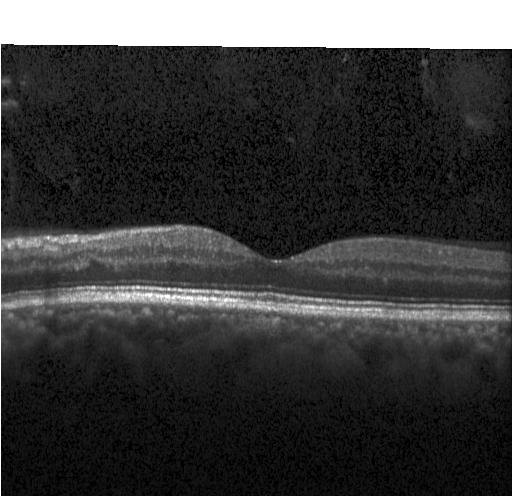

Retinal OCT B-scan — Impression: no CNV, no DME, and no drusen.